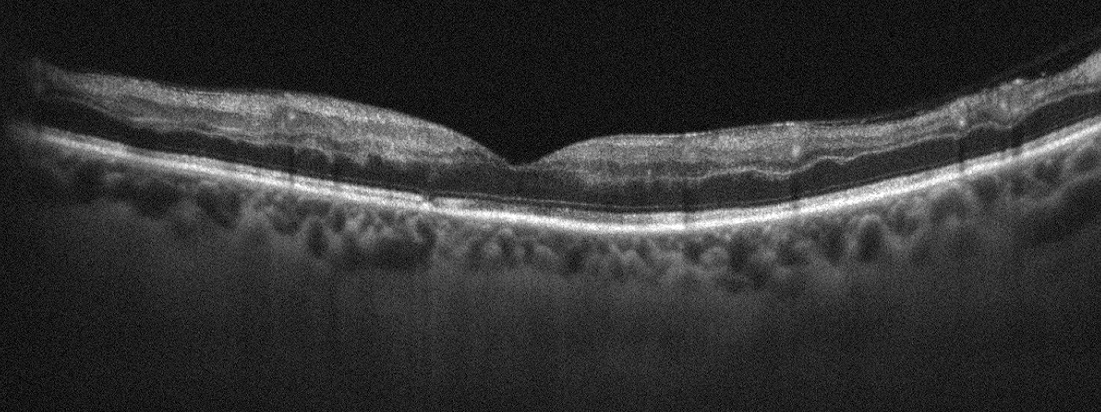 Macular scan, optical coherence tomography scan, acquired on an Optovue Avanti RTVue XR
Dx: RVO.